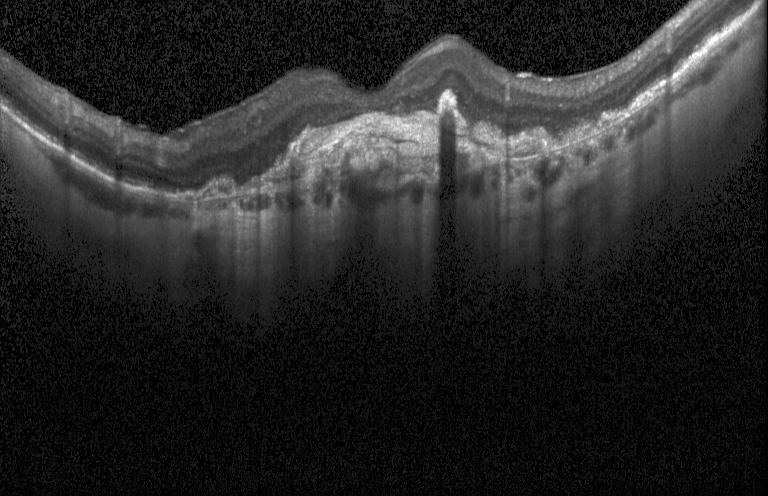 Impression: CNV.